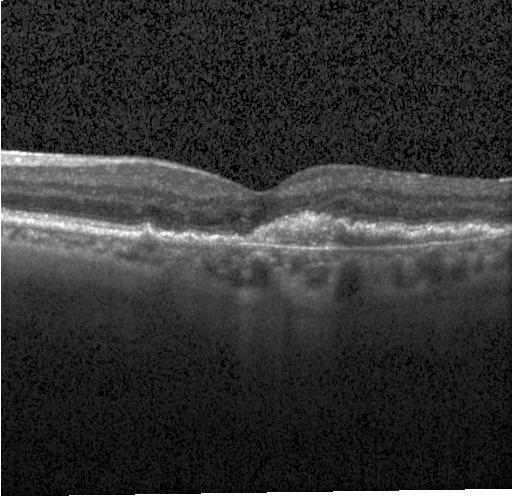
Macular OCT demonstrating choroidal neovascularization (CNV).